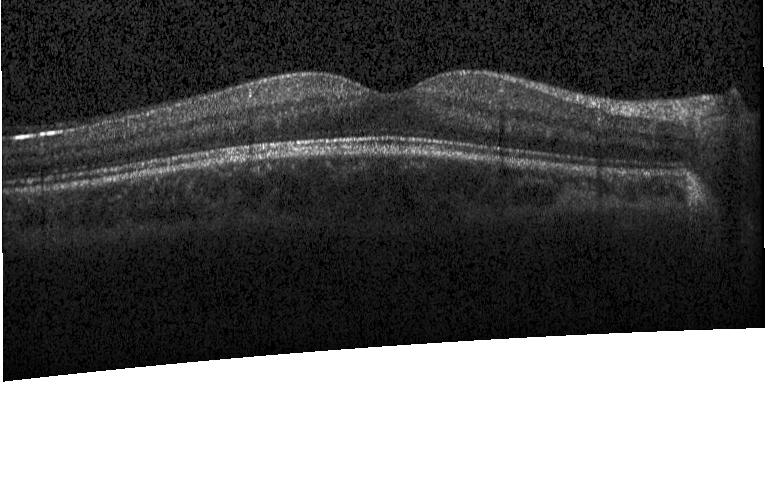 Retinal OCT B-scan
Assessment: no choroidal neovascularization, no diabetic macular edema, and no drusen.